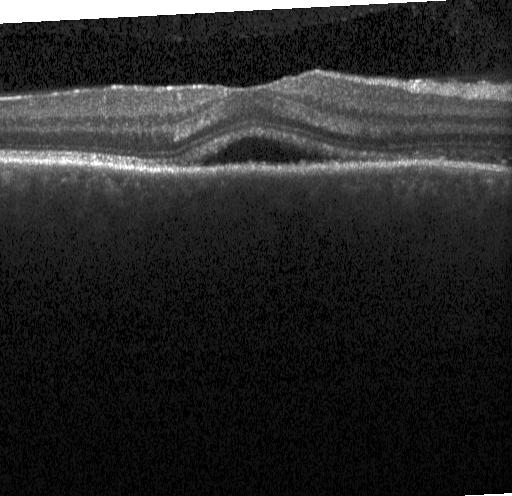
Macular OCT demonstrating CNV.